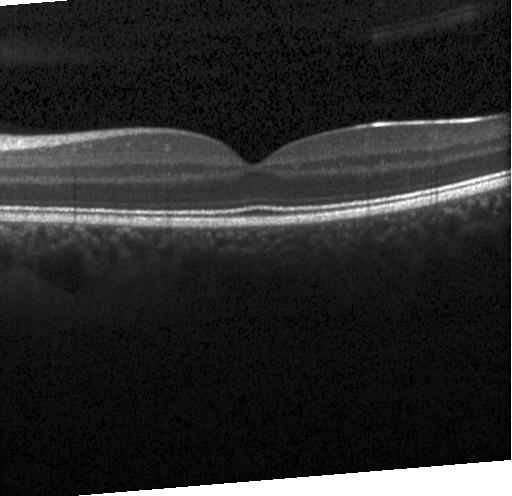
Diagnosis: no CNV, no DME, and no drusen.